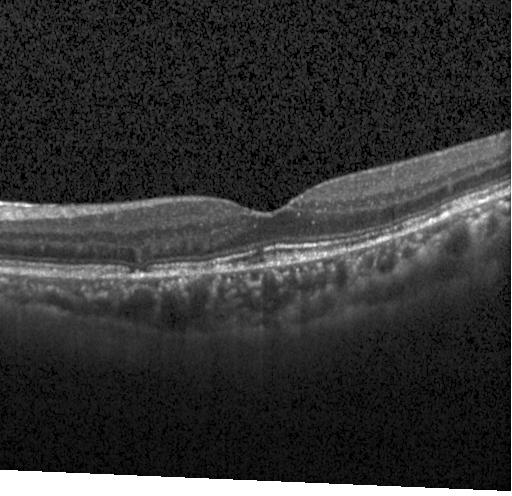
Acquired on a Heidelberg Spectralis, spectral-domain optical coherence tomography, retinal OCT B-scan. The scan shows neither choroidal neovascularization, diabetic macular edema, nor drusen.